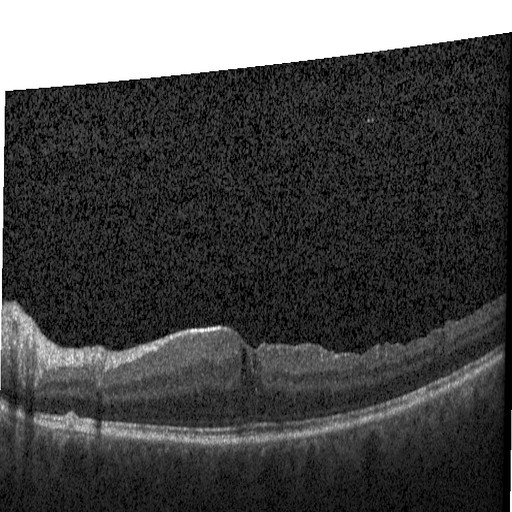

Spectral-domain OCT · OCT line scan — Diagnosis: diabetic macular edema.